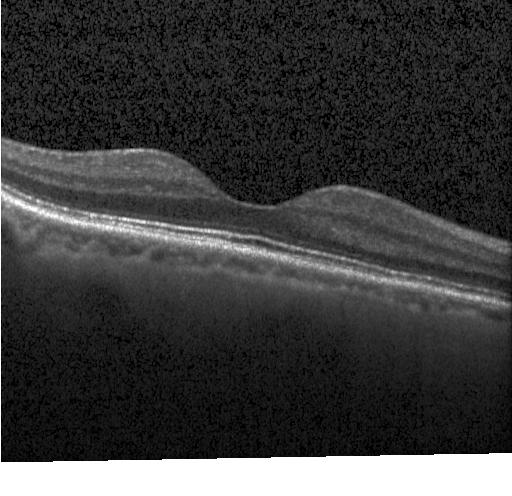
Through the macula · optical coherence tomography scan · SD-OCT · Heidelberg Spectralis
Finding: no choroidal neovascularization, diabetic macular edema, or drusen.